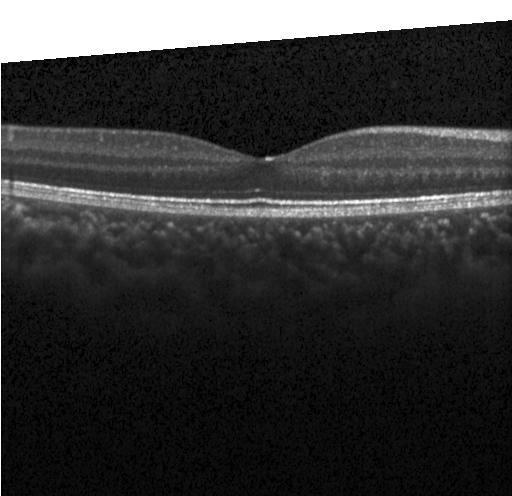

OCT scan showing neither CNV, DME, nor drusen.